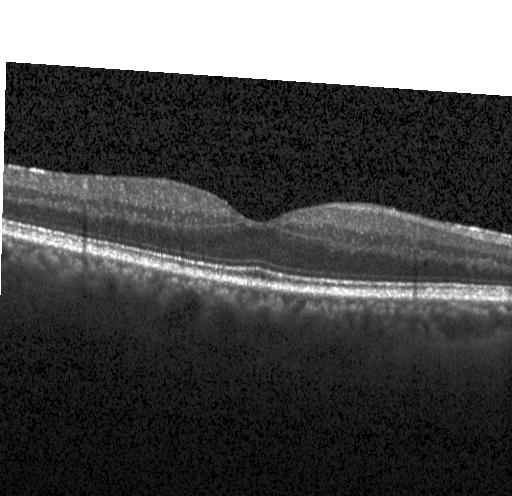 Macular OCT demonstrating no choroidal neovascularization, no diabetic macular edema, and no drusen.